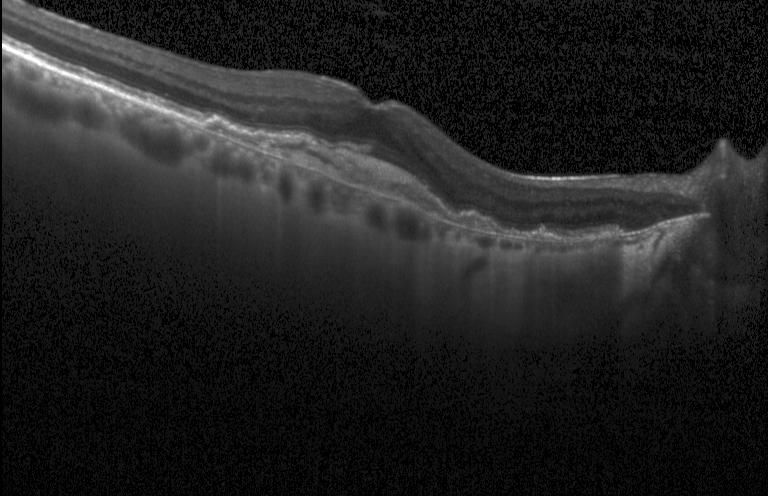 OCT B-scan — Choroidal neovascularization.